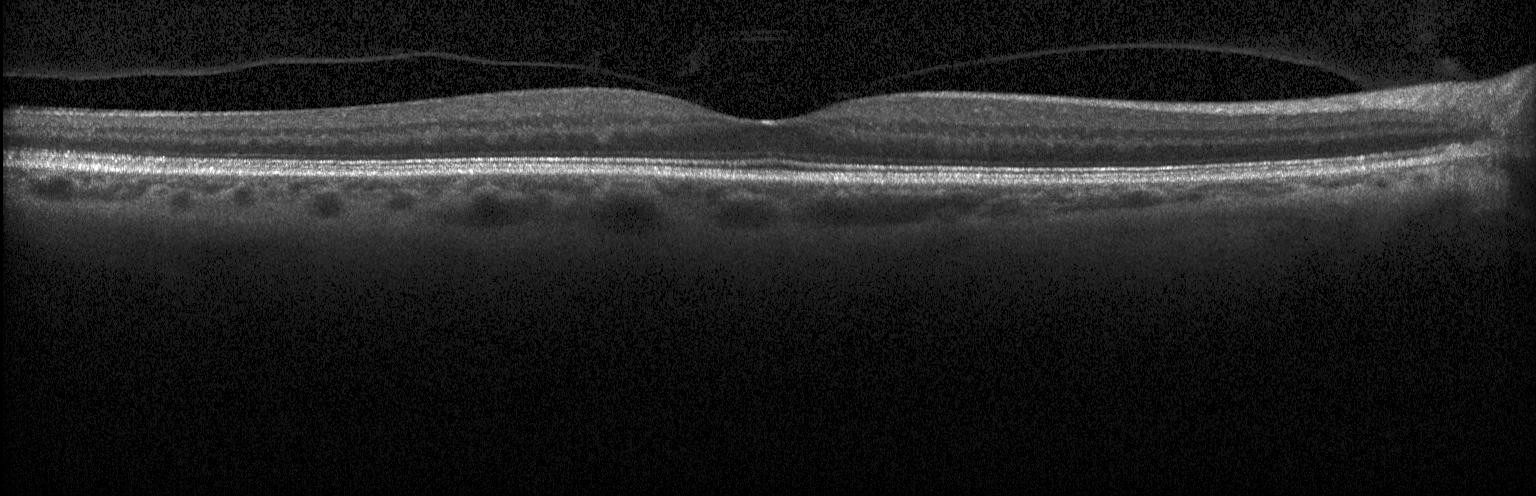

Spectral-domain OCT · optical coherence tomography B-scan — Diagnosis: neither choroidal neovascularization, diabetic macular edema, nor drusen.